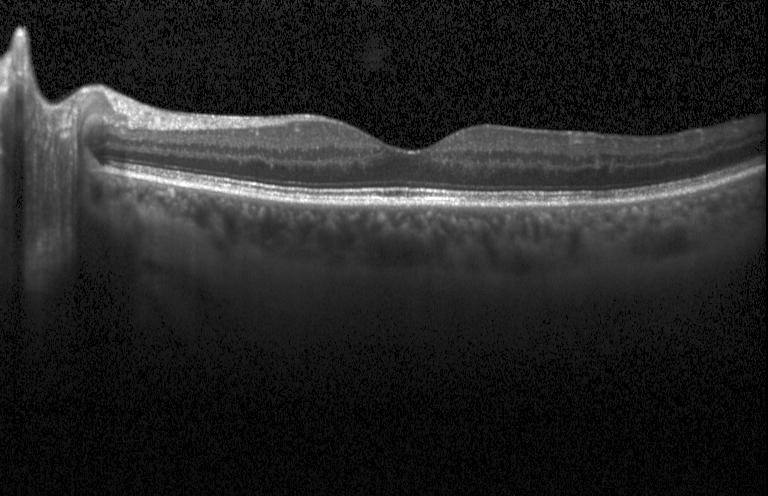

Dx: no evidence of choroidal neovascularization, diabetic macular edema, or drusen.